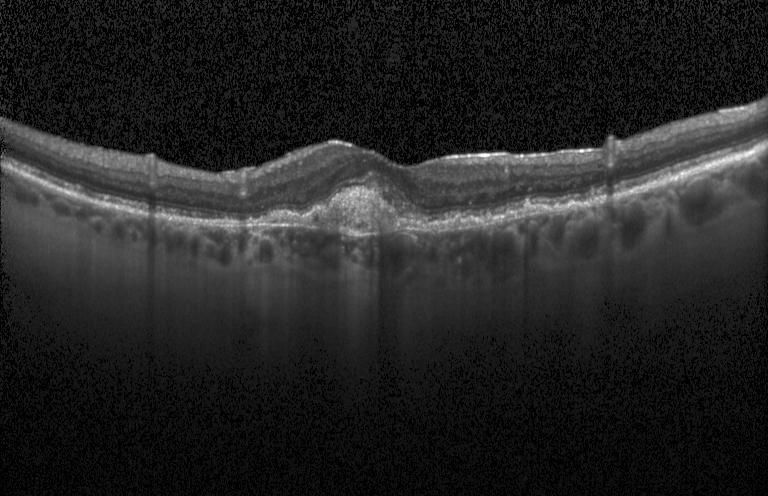 SD-OCT · horizontal scan through the fovea · retinal OCT B-scan · Heidelberg Spectralis OCT system.
Macular OCT: a choroidal neovascular membrane.